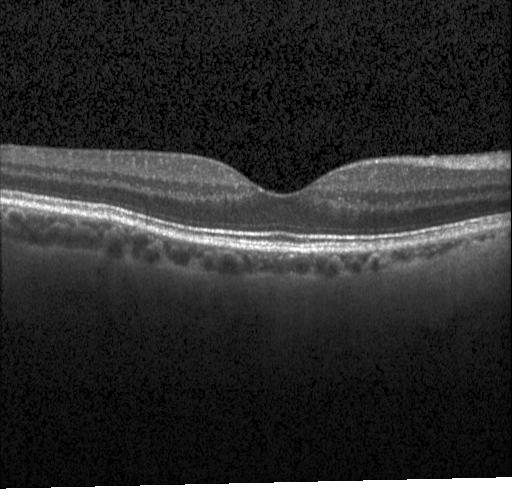

Retinal OCT cross-section
Finding: no evidence of choroidal neovascularization, diabetic macular edema, or drusen.